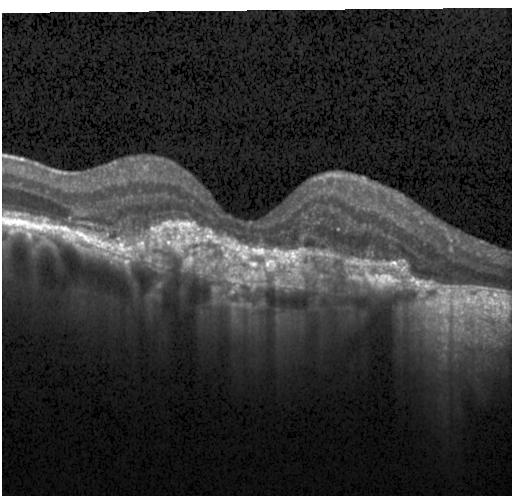

Macular OCT demonstrating a choroidal neovascular membrane.